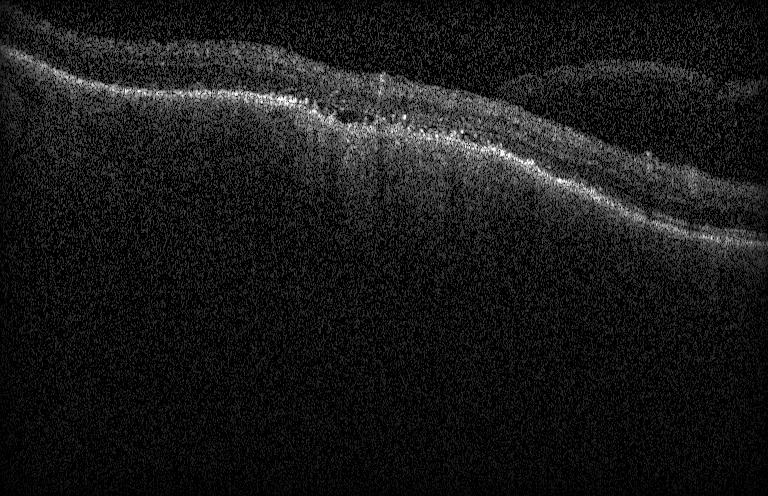
Optical coherence tomography B-scan; spectral-domain optical coherence tomography; fovea-centered.
Dx: choroidal neovascularization (CNV).